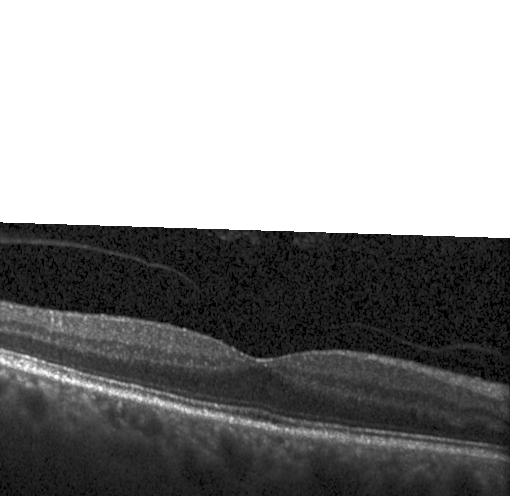

Spectral-domain optical coherence tomography, retinal OCT cross-section — OCT finding: no evidence of choroidal neovascularization, diabetic macular edema, or drusen.